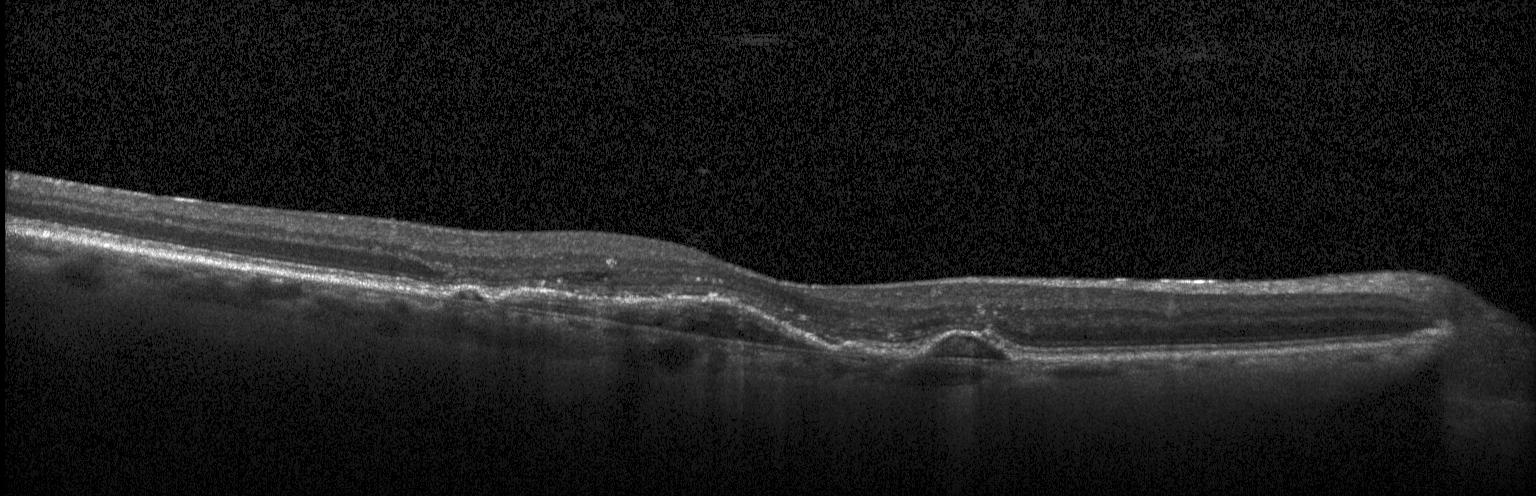 Centered on the fovea. Optical coherence tomography B-scan — Finding: a choroidal neovascular membrane.